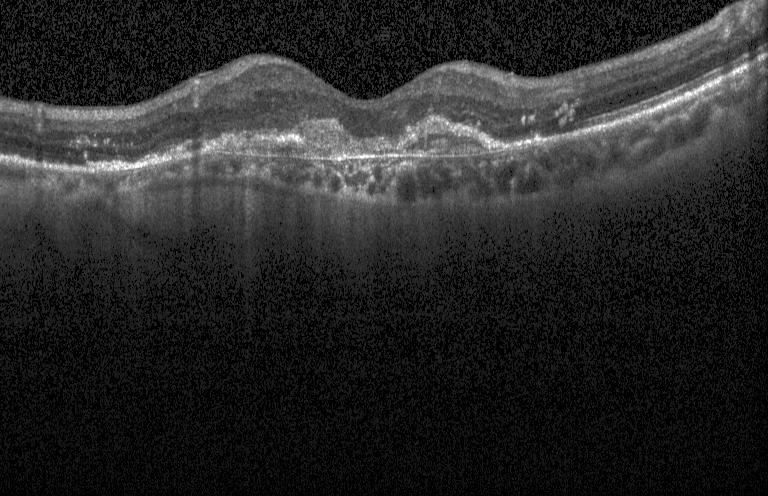
OCT finding: CNV.